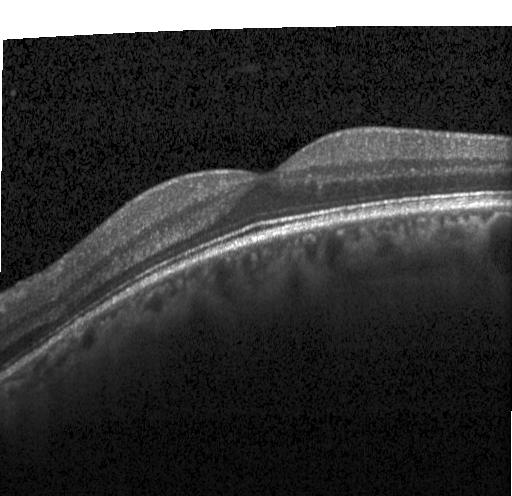 Retinal OCT B-scan · instrument: Heidelberg Spectralis · horizontal scan through the fovea · SD-OCT.
Impression: no CNV, no DME, and no drusen.